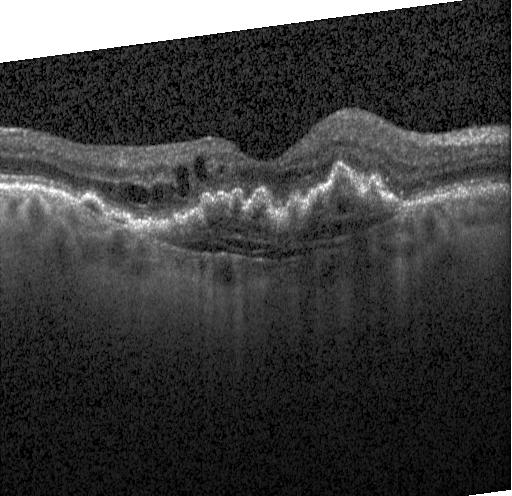 Centered on the fovea; optical coherence tomography B-scan.
Assessment: choroidal neovascularization.